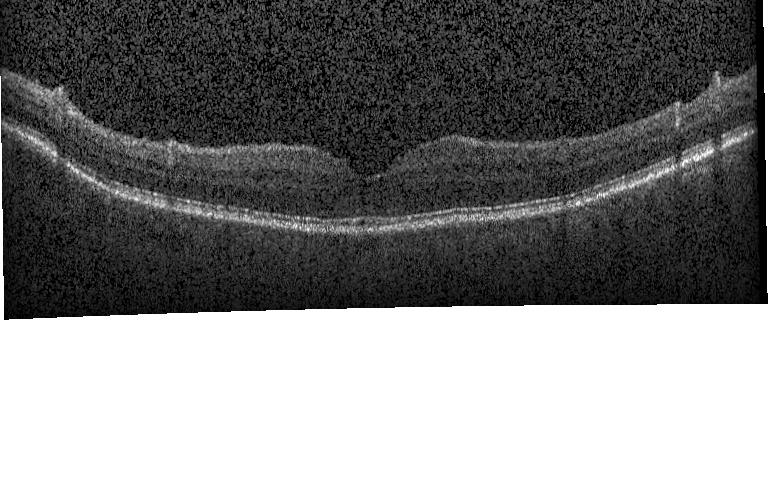
Spectral-domain OCT B-scan: no choroidal neovascularization, diabetic macular edema, or drusen.